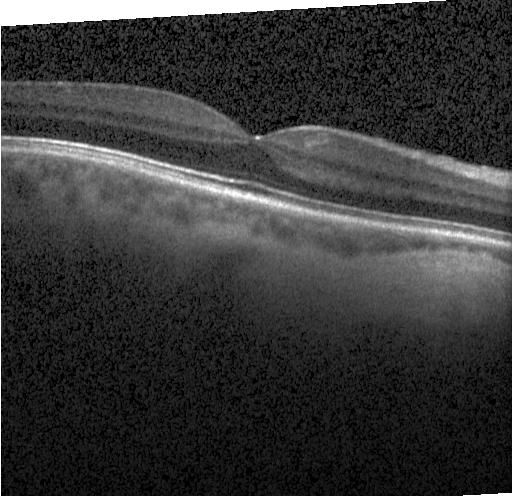 OCT finding: no choroidal neovascularization, no diabetic macular edema, and no drusen.